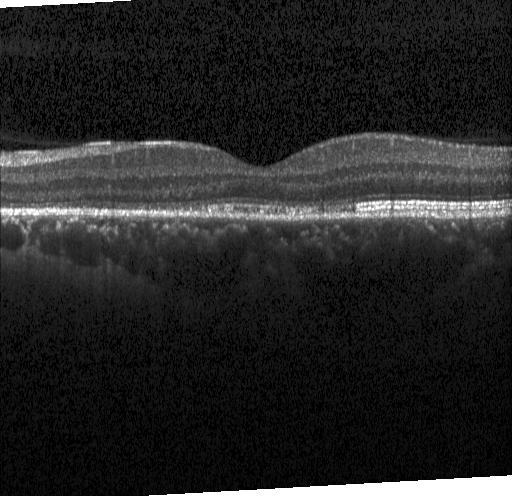
Optical coherence tomography B-scan · acquired on a Heidelberg Spectralis · fovea-centered. This B-scan demonstrates no evidence of choroidal neovascularization, diabetic macular edema, or drusen.